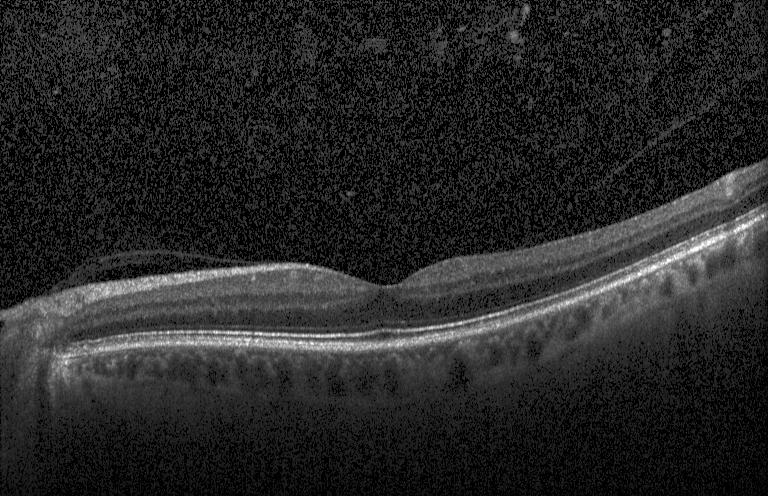 OCT B-scan. This B-scan demonstrates no CNV, no DME, and no drusen.